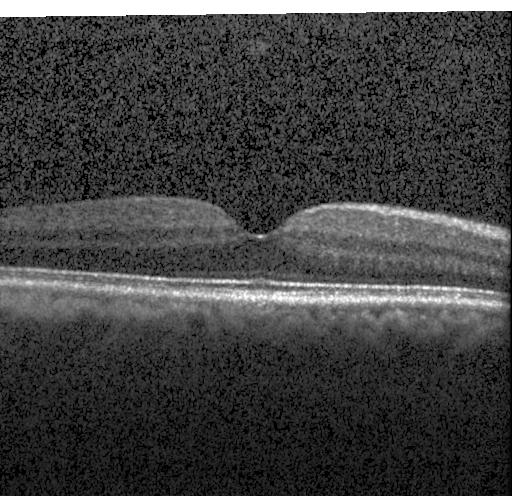 Finding: no evidence of choroidal neovascularization, diabetic macular edema, or drusen.